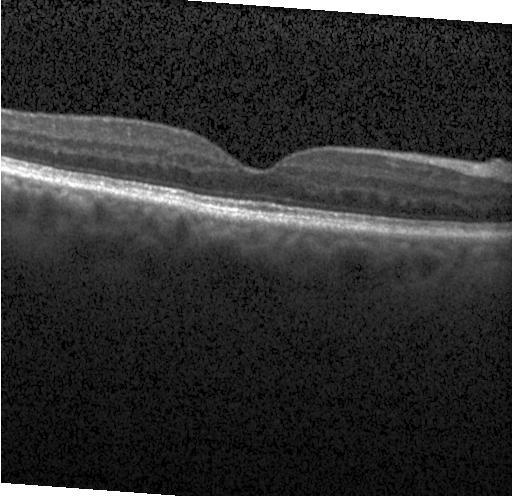 OCT finding: no choroidal neovascularization, no diabetic macular edema, and no drusen.